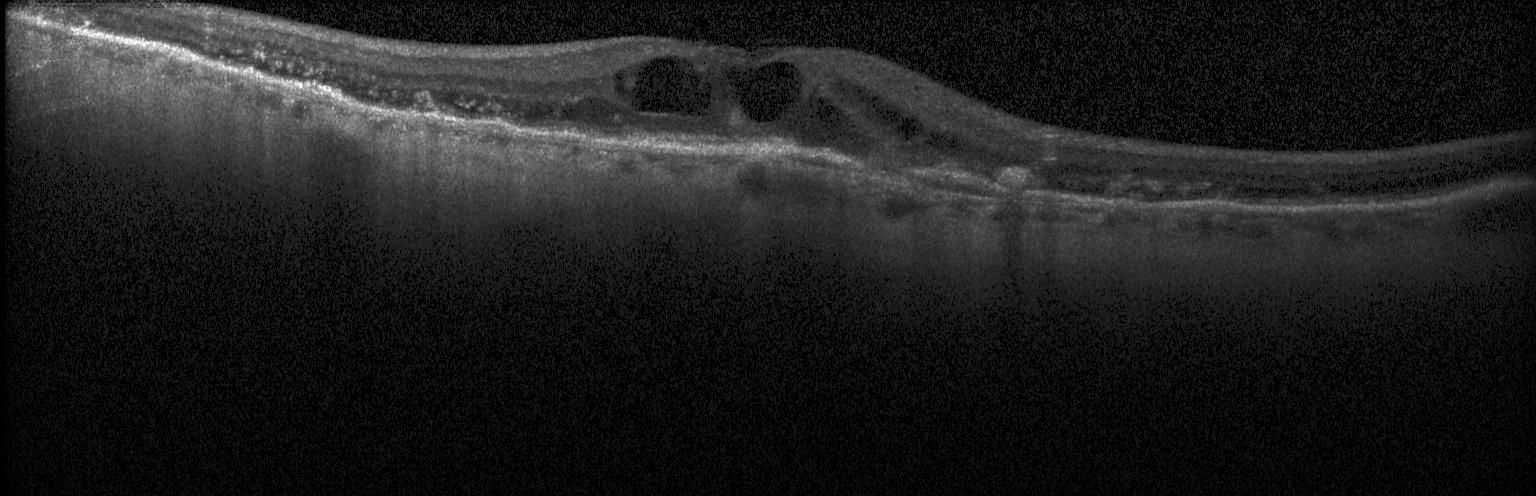

Retinal OCT B-scan.
Diagnosis: choroidal neovascularization.